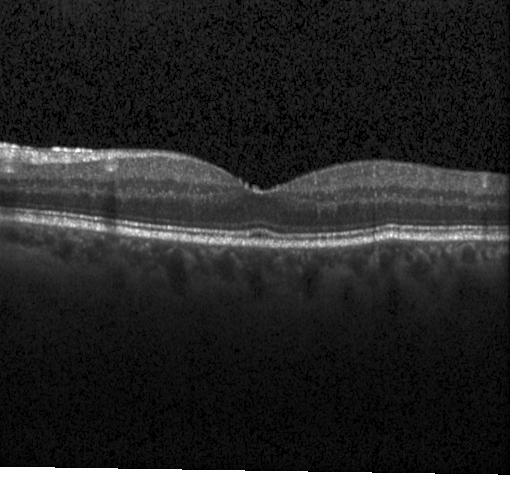
Macular scan. Retinal OCT cross-section. Heidelberg Spectralis OCT system.
Impression: no choroidal neovascularization, no diabetic macular edema, and no drusen.